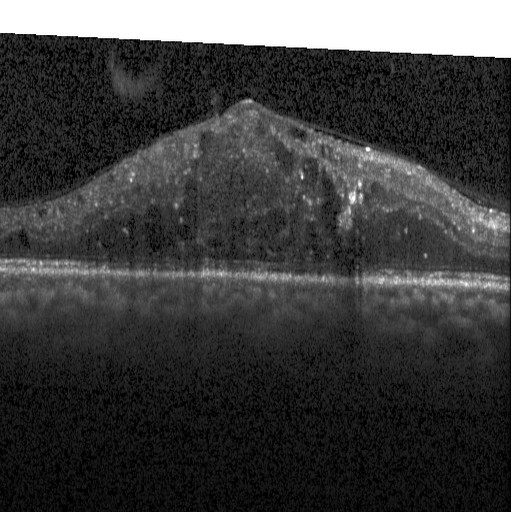 Acquired on a Heidelberg Spectralis; optical coherence tomography scan; fovea-centered; spectral-domain OCT.
Diagnosis: diabetic macular edema.